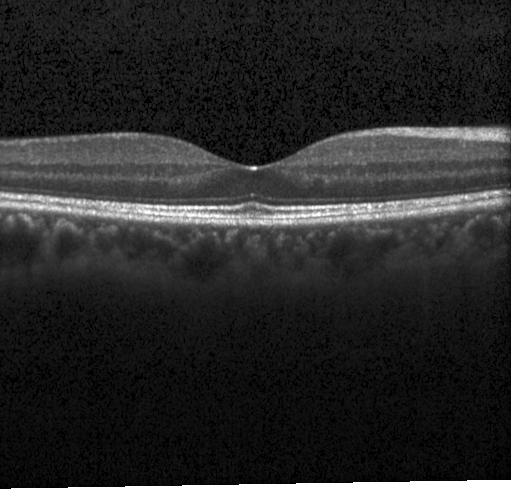

Through the macula · spectral-domain OCT · Heidelberg Spectralis · retinal OCT cross-section — Diagnosis: no choroidal neovascularization, diabetic macular edema, or drusen.